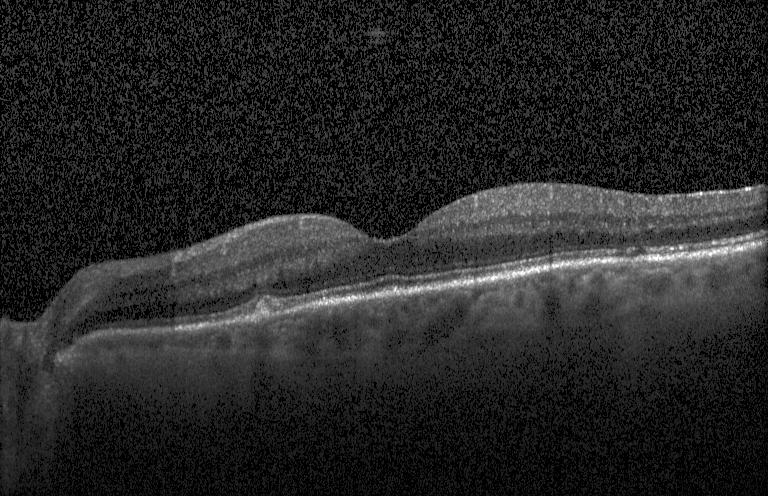

Impression: sub-RPE drusenoid deposits.